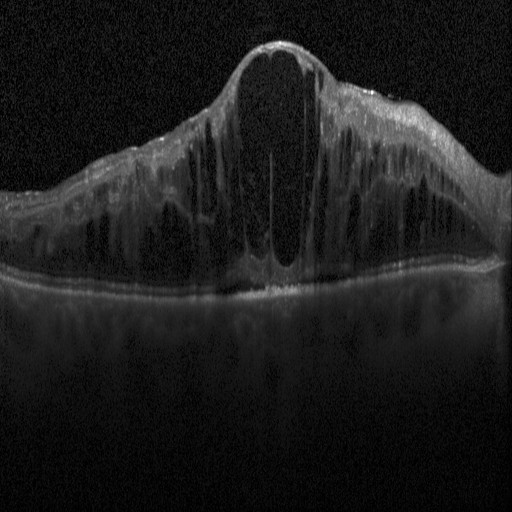 Macular OCT: DME.